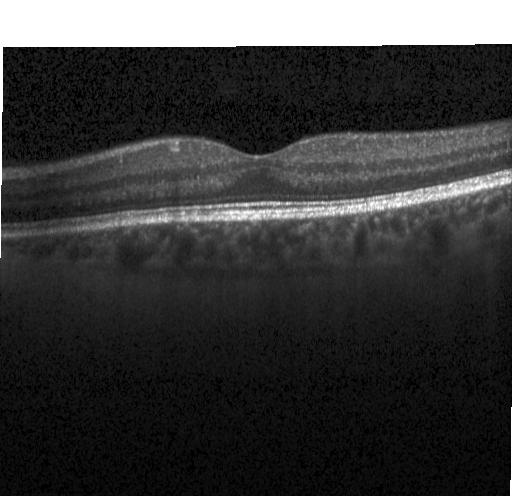

Heidelberg Spectralis OCT system. Optical coherence tomography B-scan — Assessment: neither choroidal neovascularization, diabetic macular edema, nor drusen.